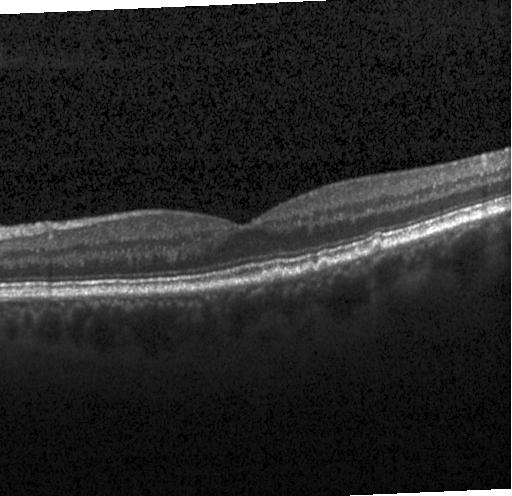 Retinal OCT B-scan
Drusen.